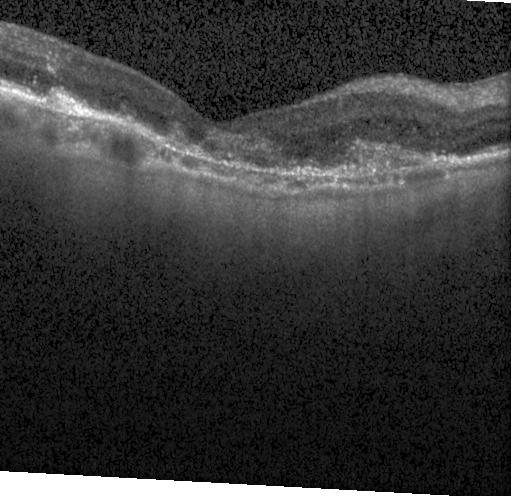
Spectral-domain optical coherence tomography · Heidelberg Spectralis · OCT B-scan
The scan shows a choroidal neovascular membrane.